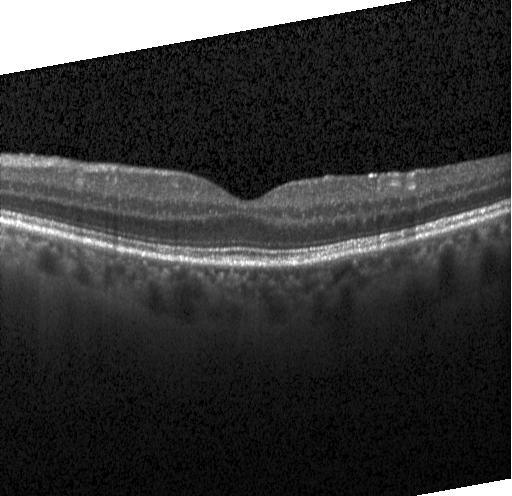
Centered on the fovea · optical coherence tomography B-scan · spectral-domain optical coherence tomography. Assessment: no CNV, no DME, and no drusen.